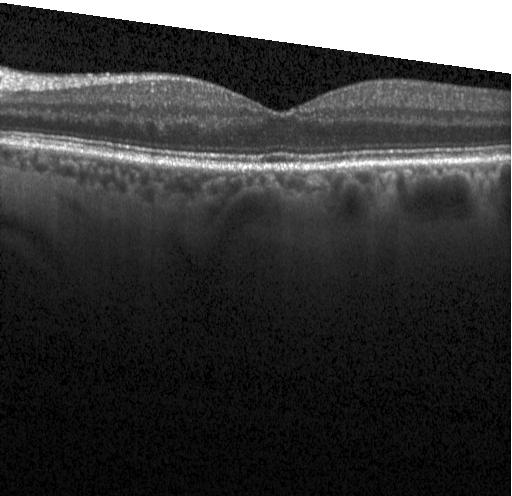
Diagnosis: no choroidal neovascularization, diabetic macular edema, or drusen.